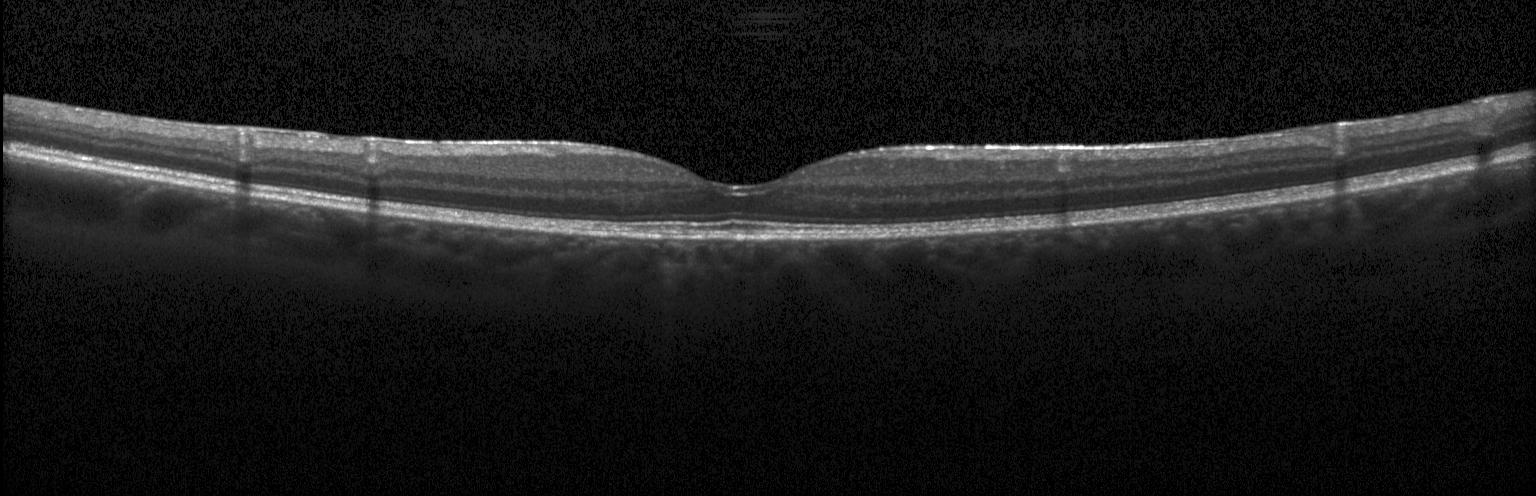

Retinal OCT B-scan, horizontal scan through the fovea, spectral-domain OCT, instrument: Heidelberg Spectralis
Finding: no choroidal neovascularization, no diabetic macular edema, and no drusen.